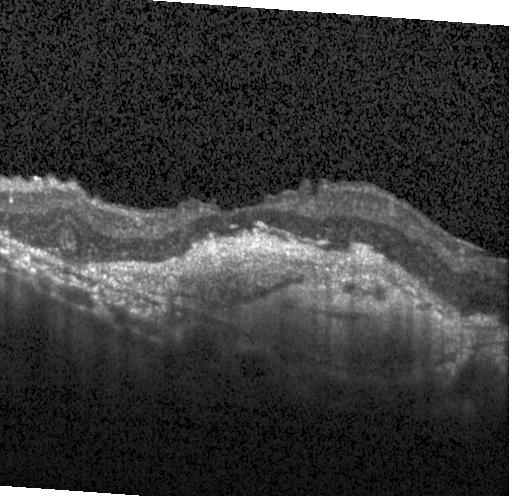

OCT B-scan · Heidelberg Spectralis · fovea-centered · spectral-domain OCT — Diagnosis: a choroidal neovascular membrane.